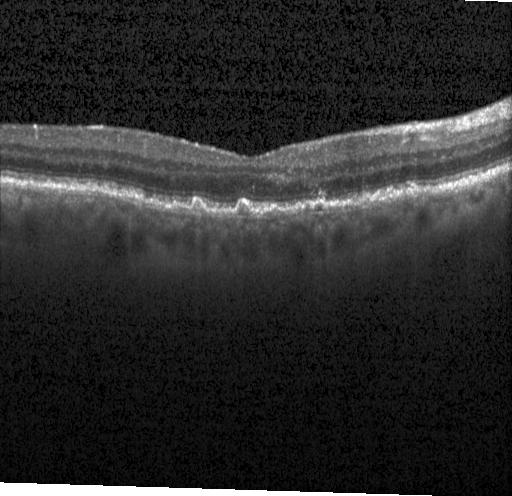

Macular OCT: sub-RPE drusenoid deposits.